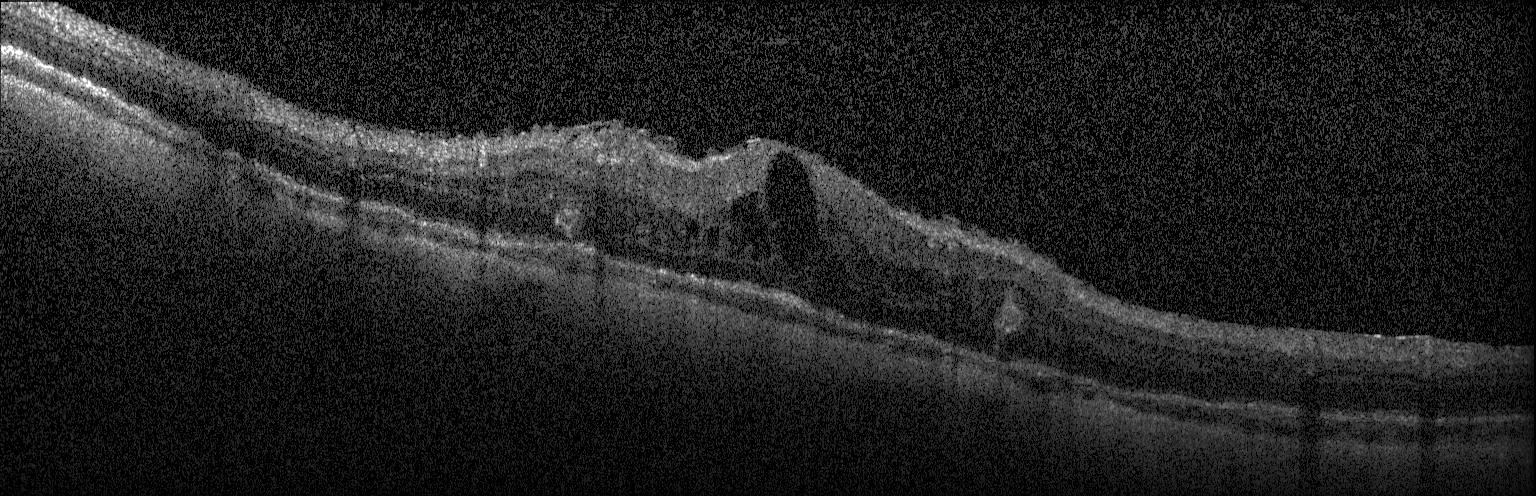

Heidelberg Spectralis OCT system. Spectral-domain OCT. Centered on the fovea. OCT line scan.
Impression: diabetic macular edema (DME).